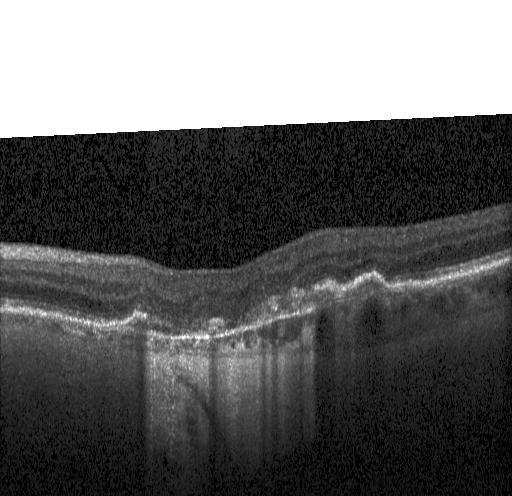
Dx: a choroidal neovascular membrane.